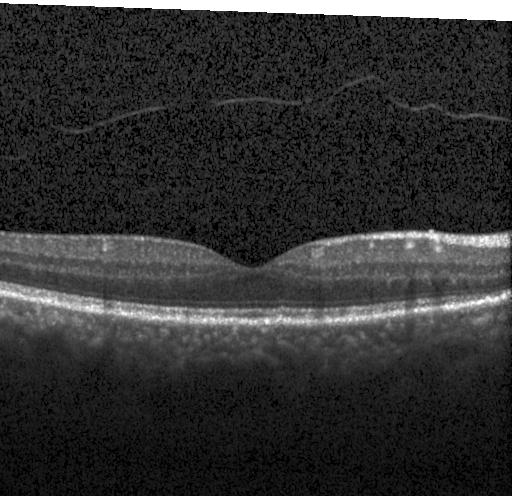
Heidelberg Spectralis. Optical coherence tomography B-scan. Impression: no evidence of choroidal neovascularization, diabetic macular edema, or drusen.